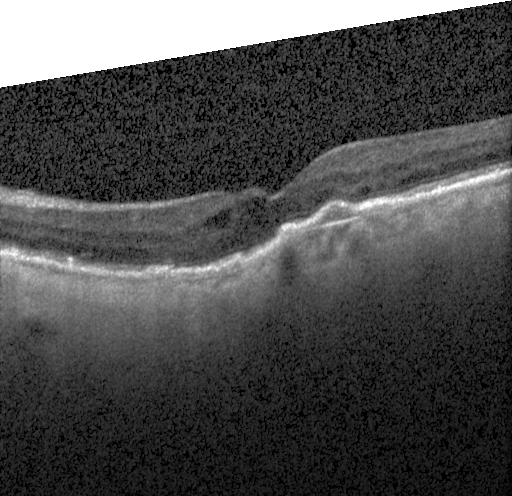
This B-scan demonstrates a choroidal neovascular membrane.